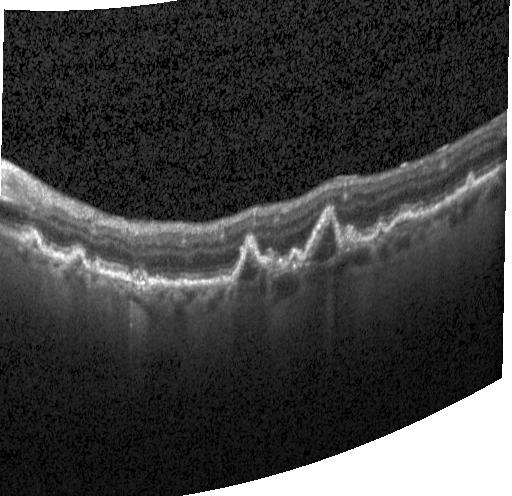 Optical coherence tomography scan; macular scan — Finding: a choroidal neovascular membrane.